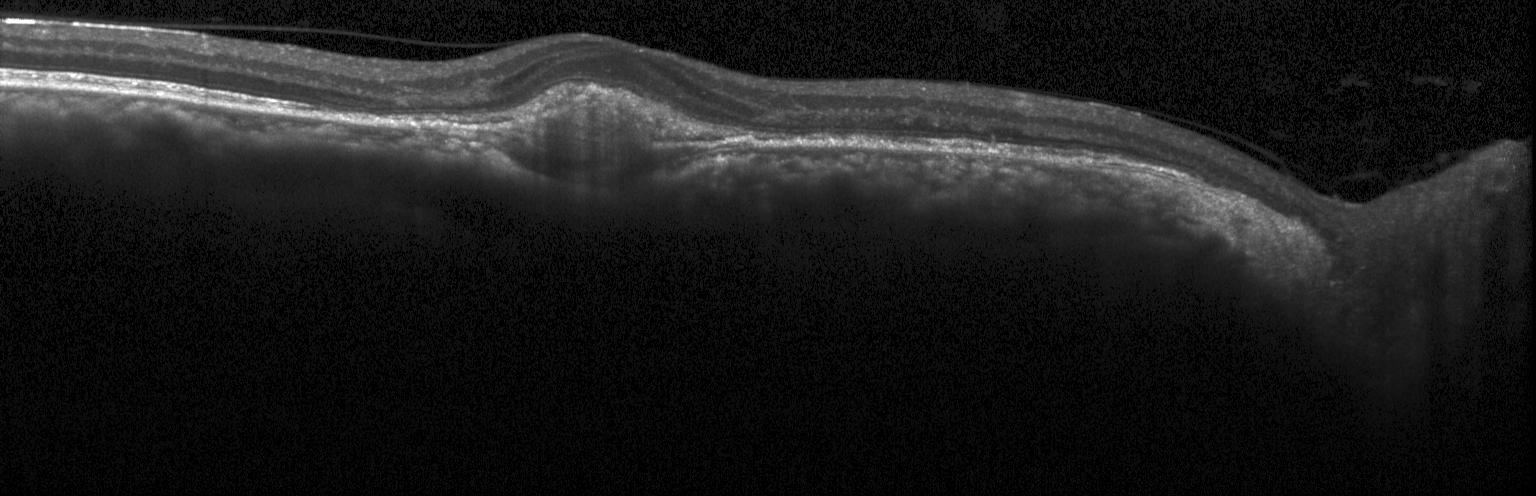
Finding: a choroidal neovascular membrane.